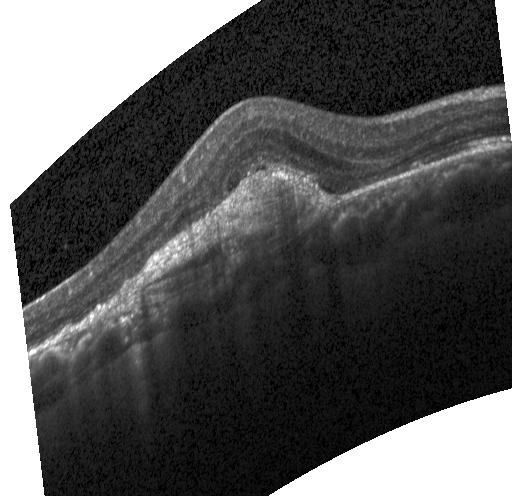
Through the macula · optical coherence tomography B-scan · spectral-domain optical coherence tomography · Heidelberg Spectralis OCT system
The scan shows CNV.